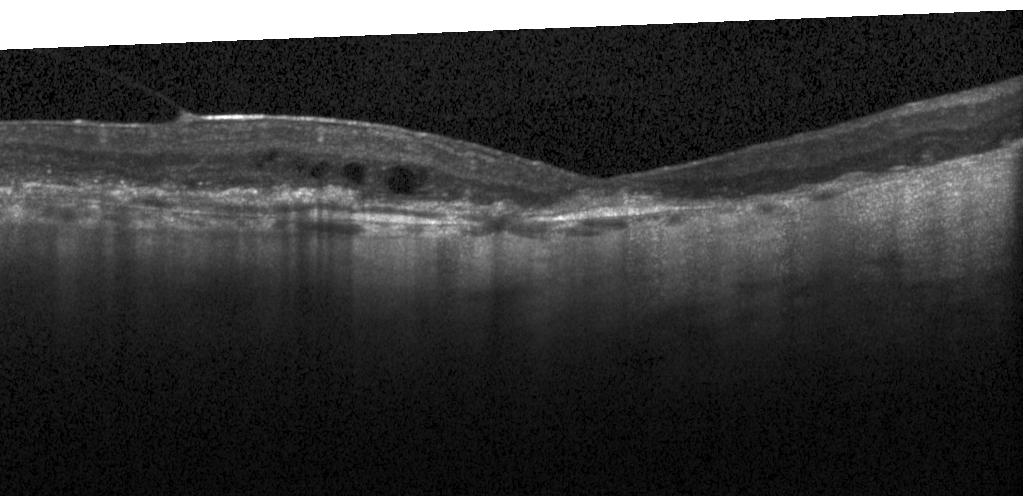

Optical coherence tomography B-scan; Heidelberg Spectralis OCT system — Finding: choroidal neovascularization.